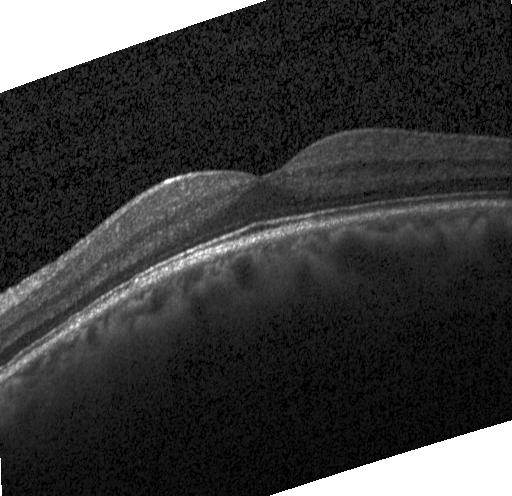 Spectral-domain optical coherence tomography, acquired on a Heidelberg Spectralis, retinal OCT B-scan
Dx: neither choroidal neovascularization, diabetic macular edema, nor drusen.